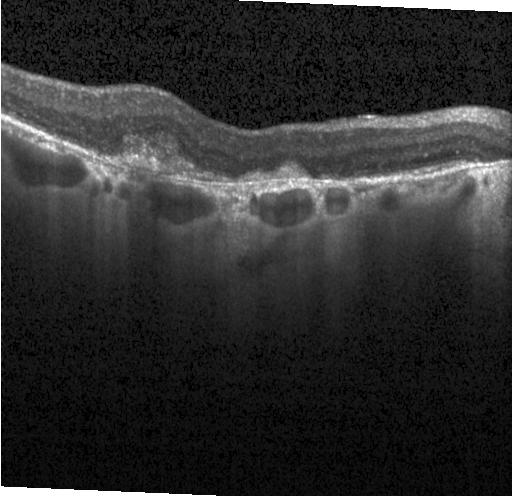
Optical coherence tomography scan. Impression: a choroidal neovascular membrane.